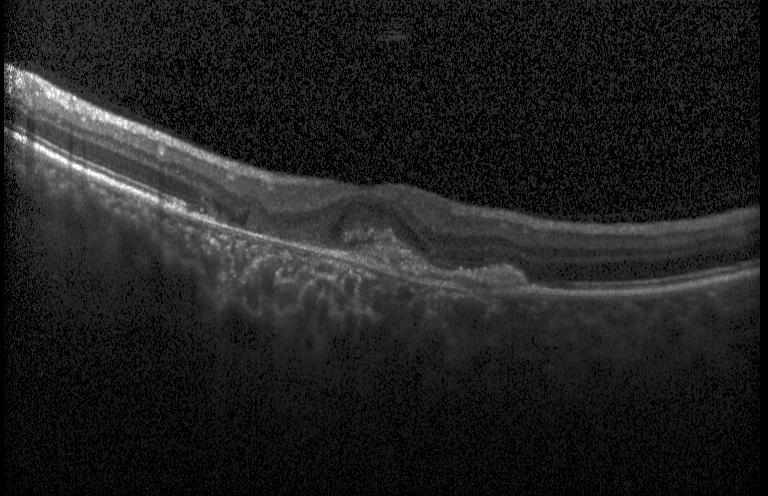 Impression: choroidal neovascularization (CNV).